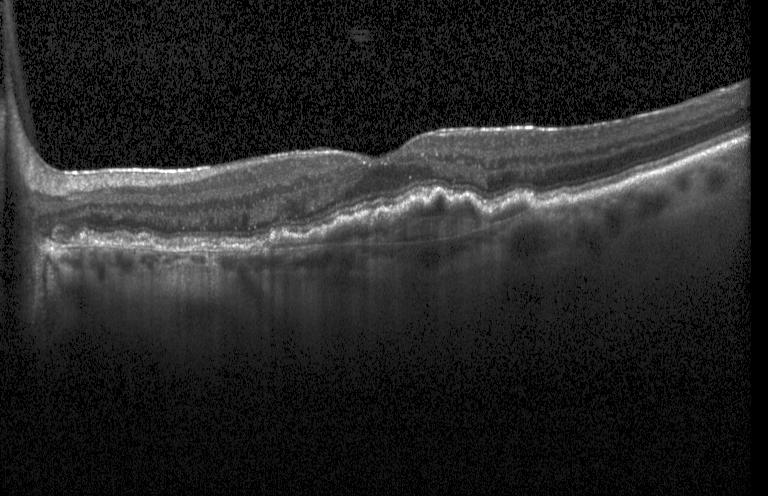 Optical coherence tomography B-scan. Spectral-domain optical coherence tomography — The scan shows a choroidal neovascular membrane.